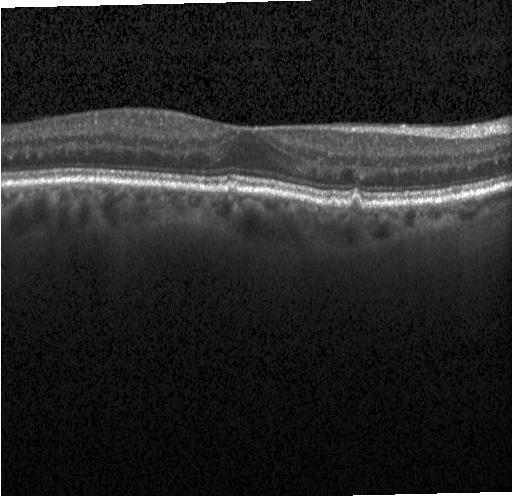
OCT finding: drusen.